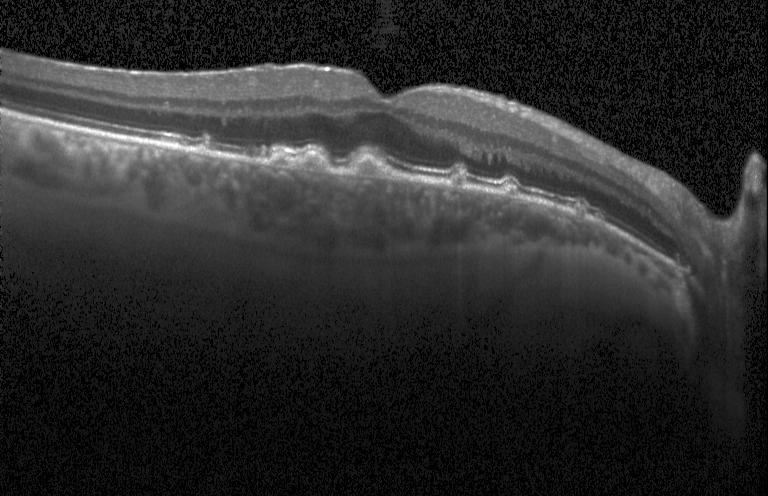

Impression: sub-RPE drusenoid deposits.